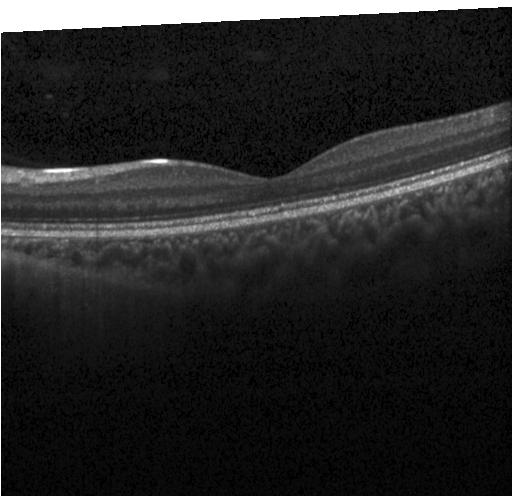

Diagnosis: no CNV, DME, or drusen.